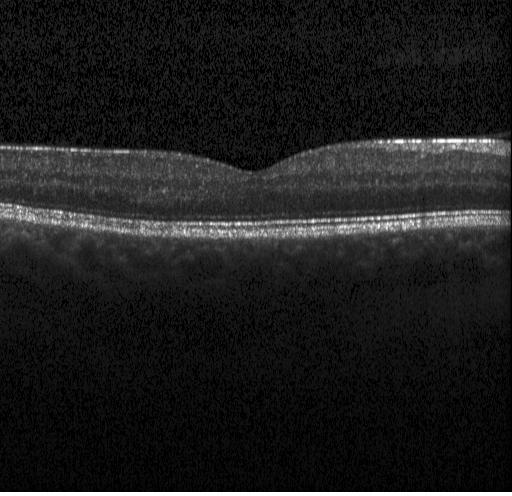
OCT line scan; SD-OCT — Finding: no choroidal neovascularization, no diabetic macular edema, and no drusen.